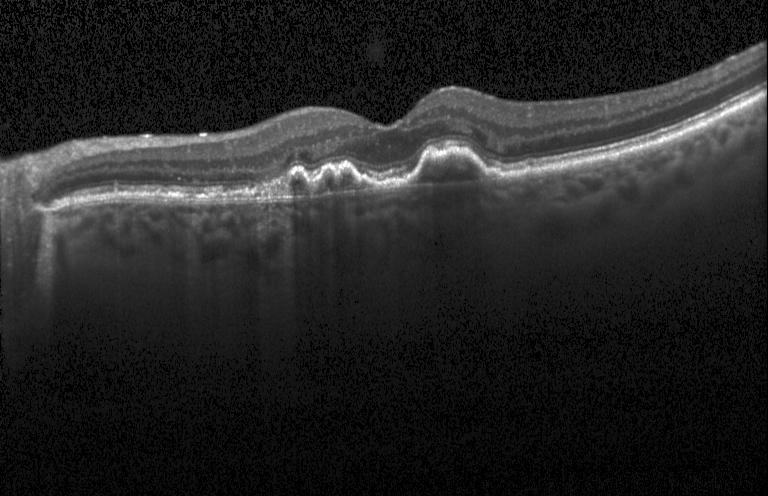 Instrument: Heidelberg Spectralis, retinal OCT B-scan, macular scan, spectral-domain OCT
This B-scan demonstrates CNV.